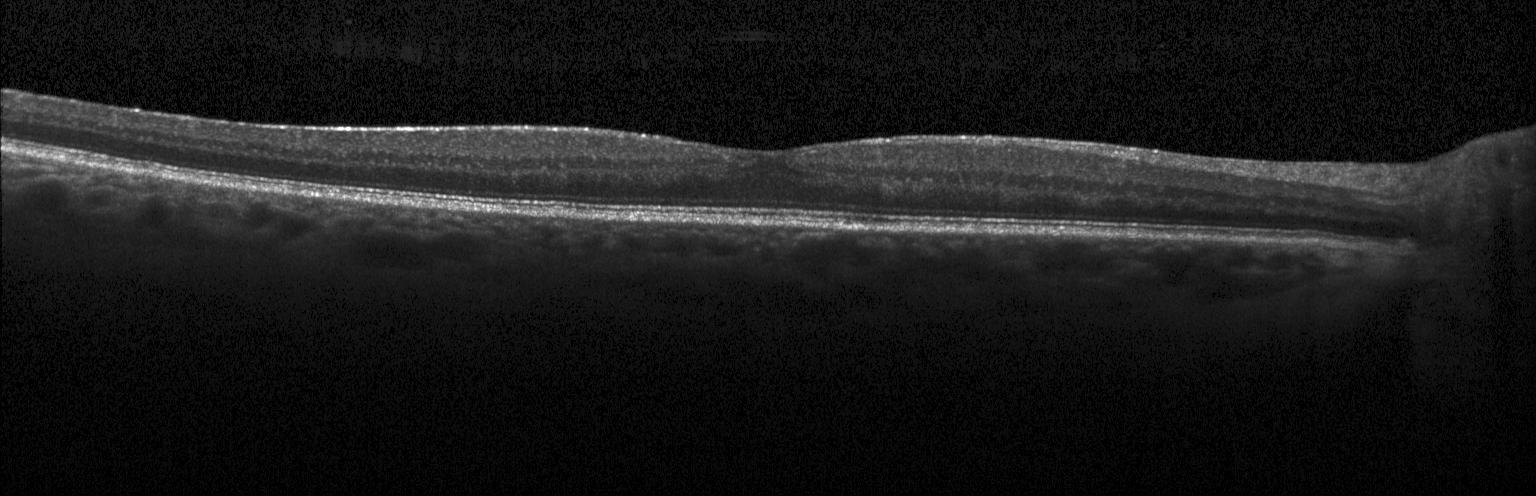 Heidelberg Spectralis · retinal OCT B-scan
Assessment: no evidence of choroidal neovascularization, diabetic macular edema, or drusen.